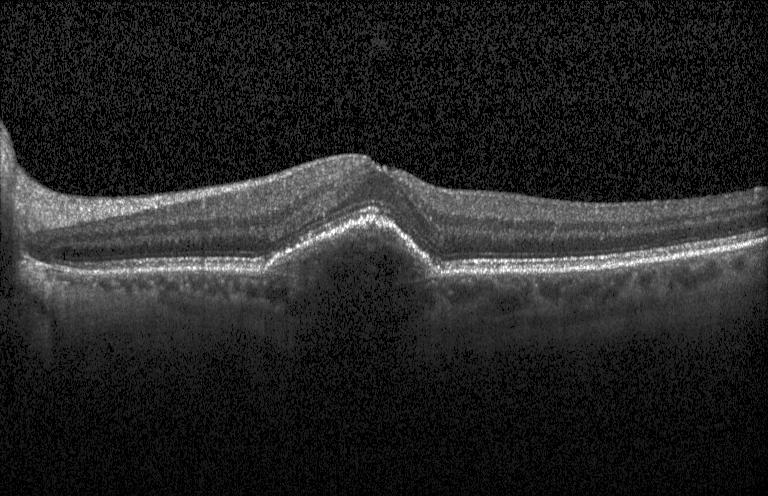
OCT B-scan. Heidelberg Spectralis OCT system. Spectral-domain OCT
Impression: a choroidal neovascular membrane.